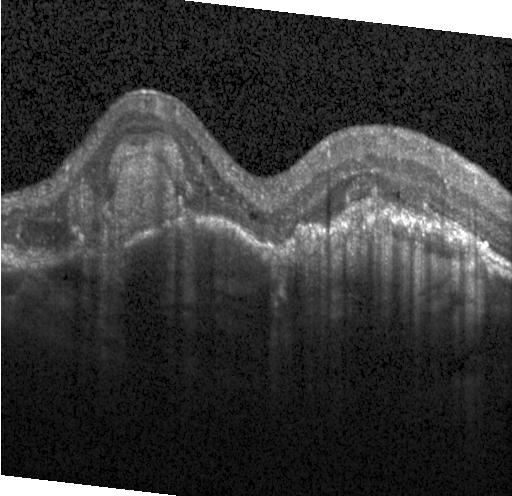

Diagnosis: a choroidal neovascular membrane.